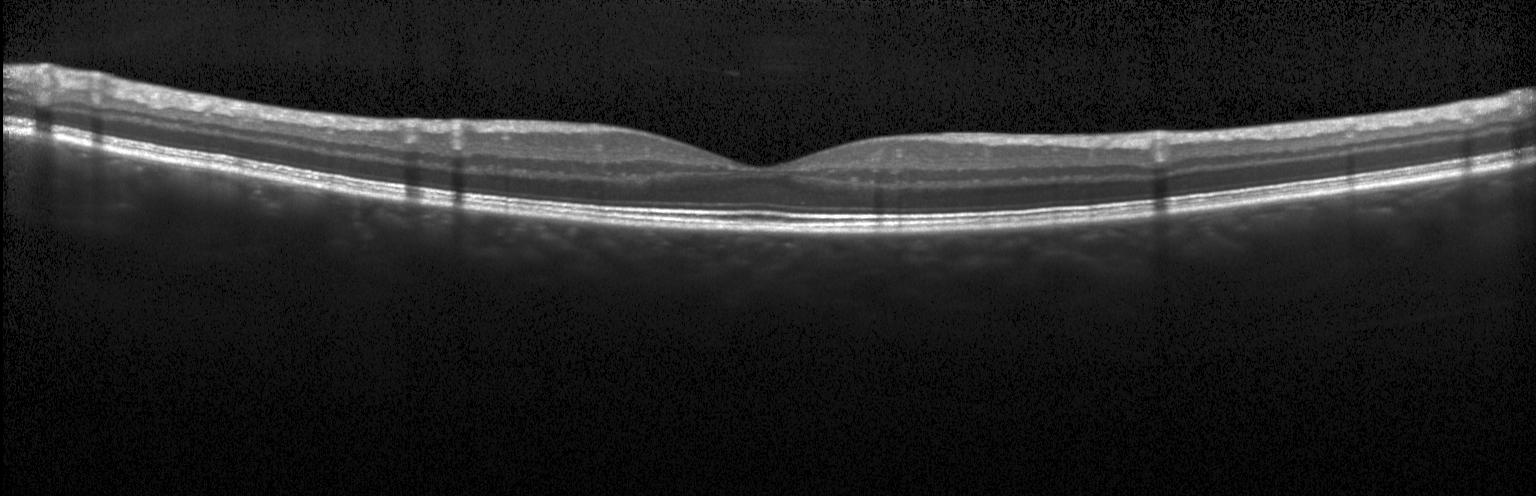
Fovea-centered; optical coherence tomography scan; SD-OCT; Heidelberg Spectralis OCT system
This B-scan demonstrates no evidence of choroidal neovascularization, diabetic macular edema, or drusen.